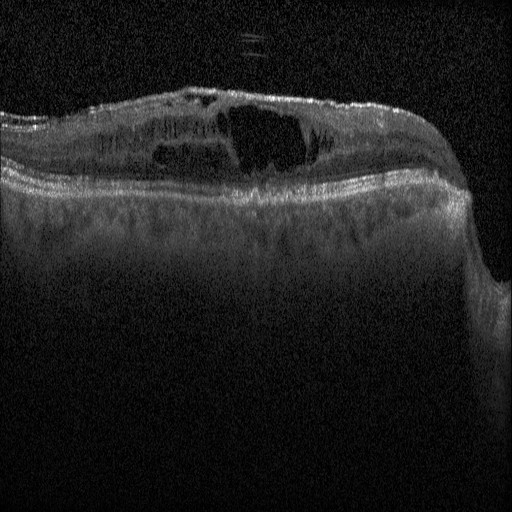
Retinal OCT B-scan; horizontal scan through the fovea; SD-OCT
Diagnosis: diabetic macular edema.